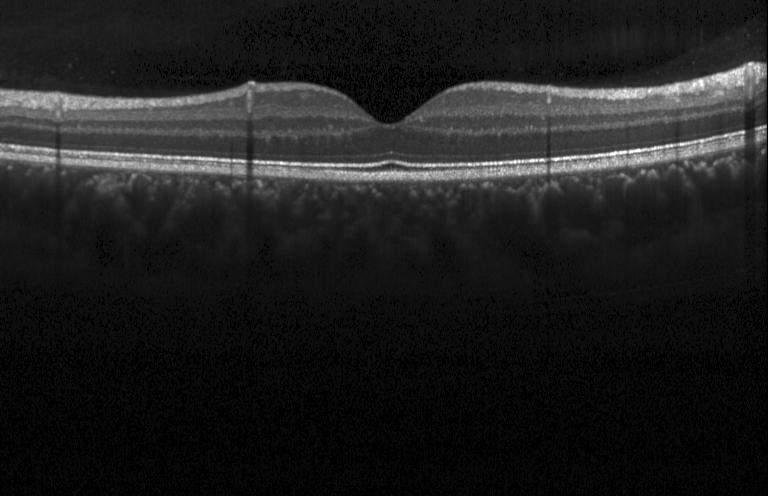

Acquired on a Heidelberg Spectralis; spectral-domain OCT; retinal OCT B-scan — OCT finding: no choroidal neovascularization, no diabetic macular edema, and no drusen.